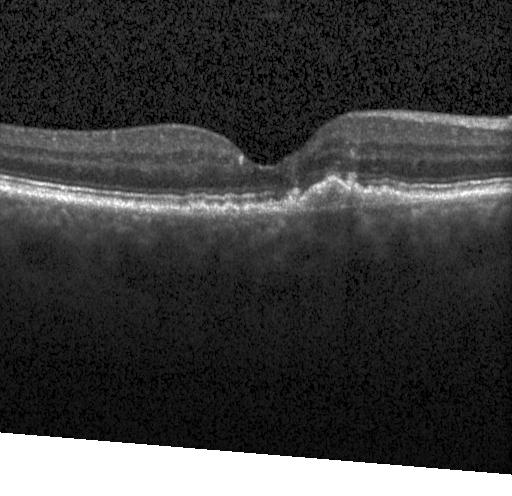 Retinal OCT B-scan. Fovea-centered. Instrument: Heidelberg Spectralis.
Impression: choroidal neovascularization.